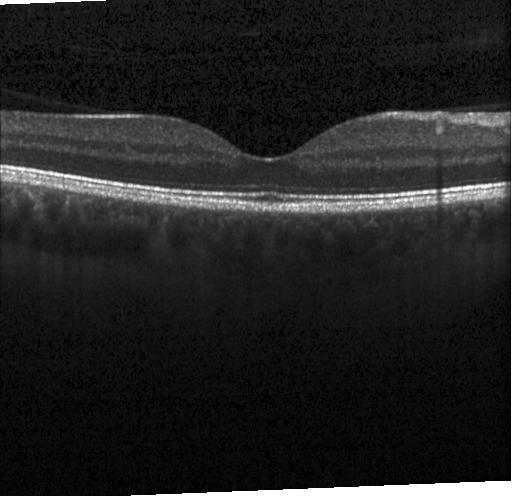

Optical coherence tomography B-scan.
Finding: no evidence of choroidal neovascularization, diabetic macular edema, or drusen.